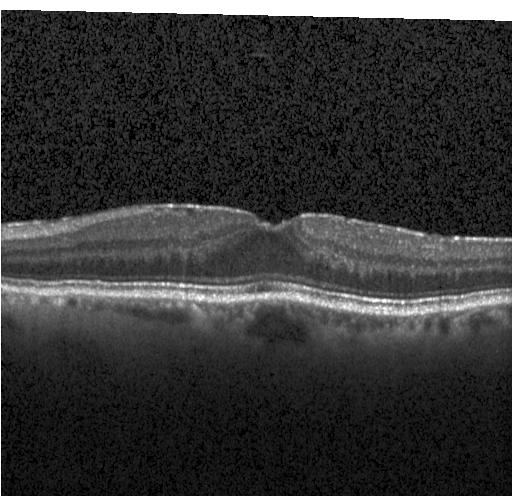
Fovea-centered, optical coherence tomography B-scan — Diagnosis: no evidence of choroidal neovascularization, diabetic macular edema, or drusen.